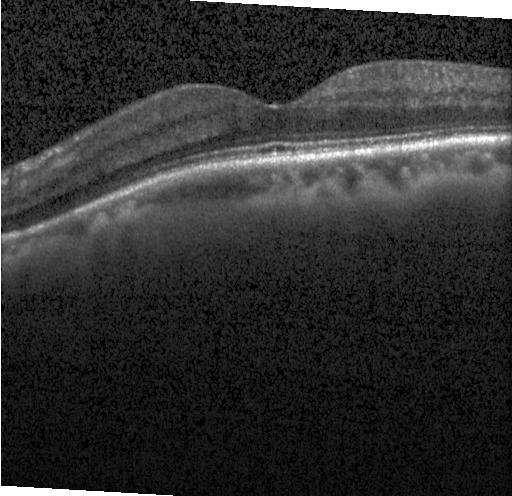 Optical coherence tomography B-scan; centered on the fovea. This B-scan demonstrates neither choroidal neovascularization, diabetic macular edema, nor drusen.